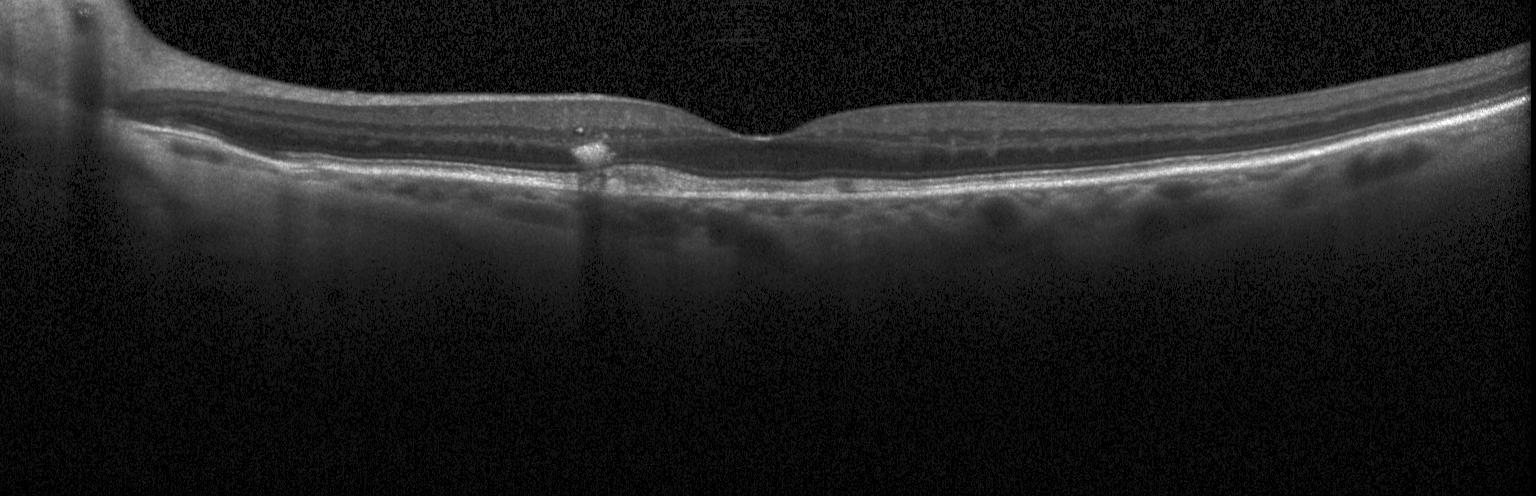 Spectral-domain OCT, OCT line scan, through the macula
Macular OCT: multiple drusen.